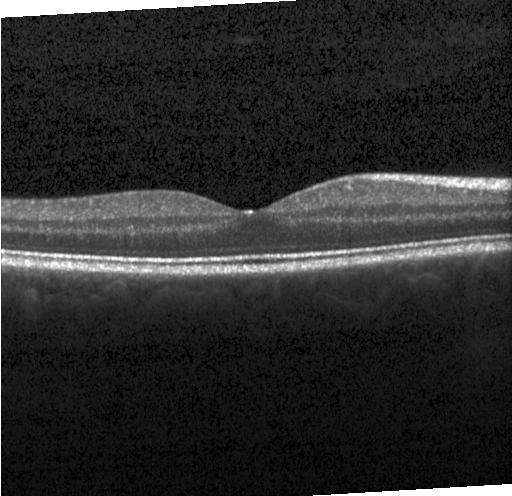

Retinal OCT cross-section. No choroidal neovascularization, diabetic macular edema, or drusen.